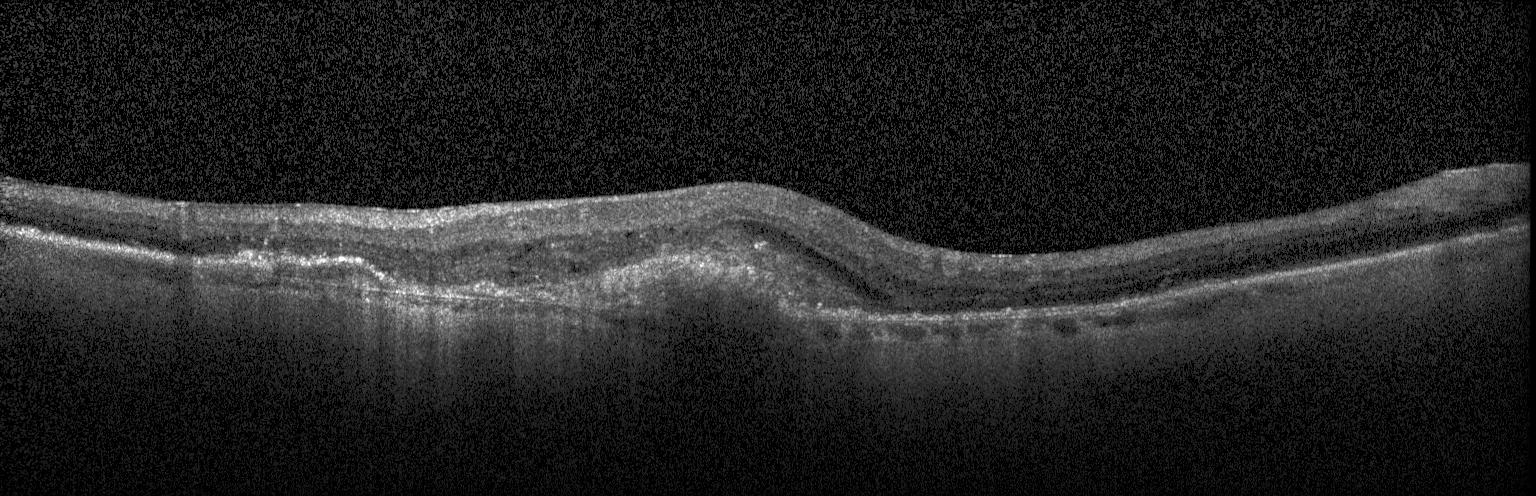 Macular OCT: a choroidal neovascular membrane.